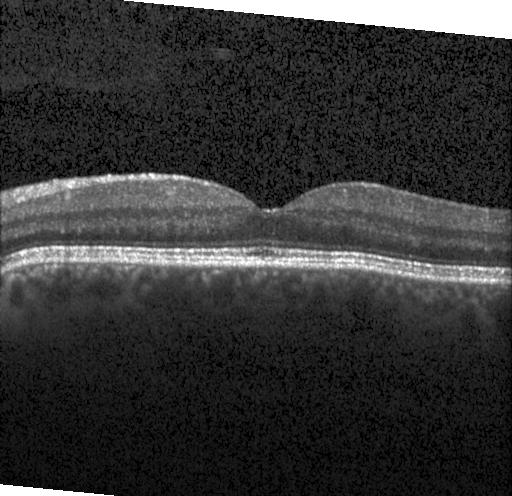 OCT line scan · macular scan. This B-scan demonstrates neither choroidal neovascularization, diabetic macular edema, nor drusen.